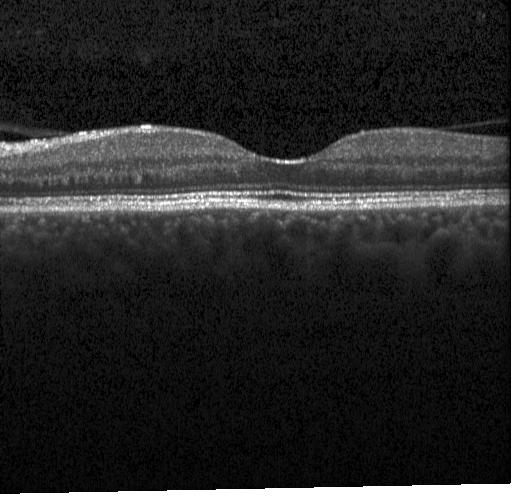

Retinal OCT B-scan. Dx: no evidence of CNV, DME, or drusen.